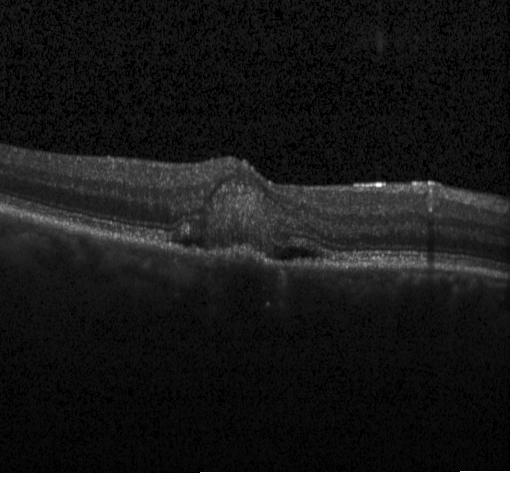 Impression: CNV.